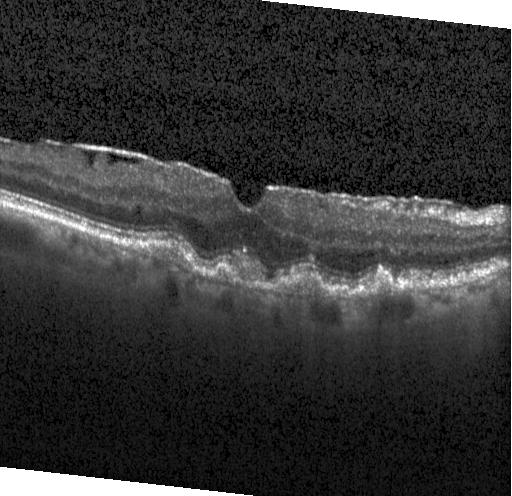

Impression: sub-RPE drusenoid deposits.